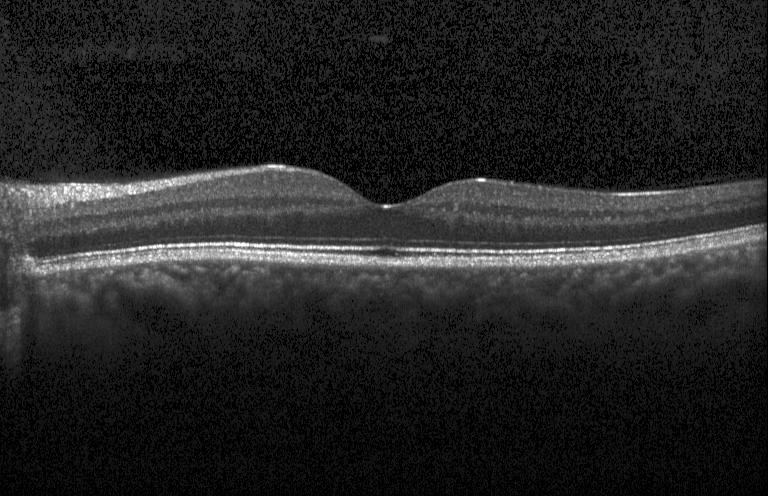

OCT finding: neither CNV, DME, nor drusen.